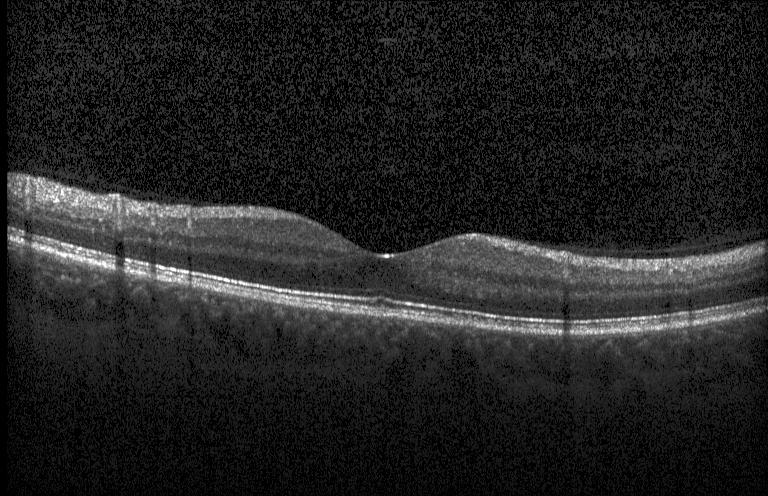 Retinal OCT B-scan. Impression: no choroidal neovascularization, no diabetic macular edema, and no drusen.